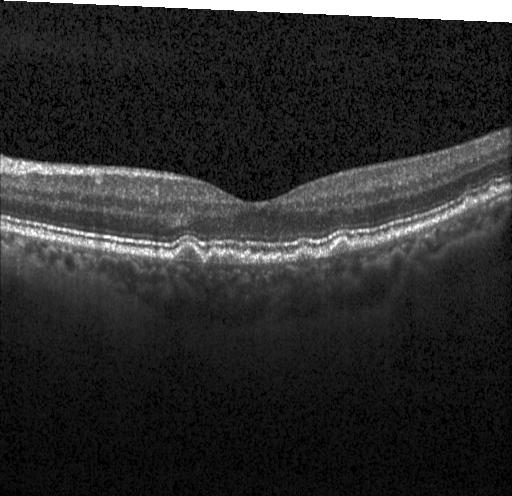 Centered on the fovea; optical coherence tomography scan — Finding: multiple drusen.